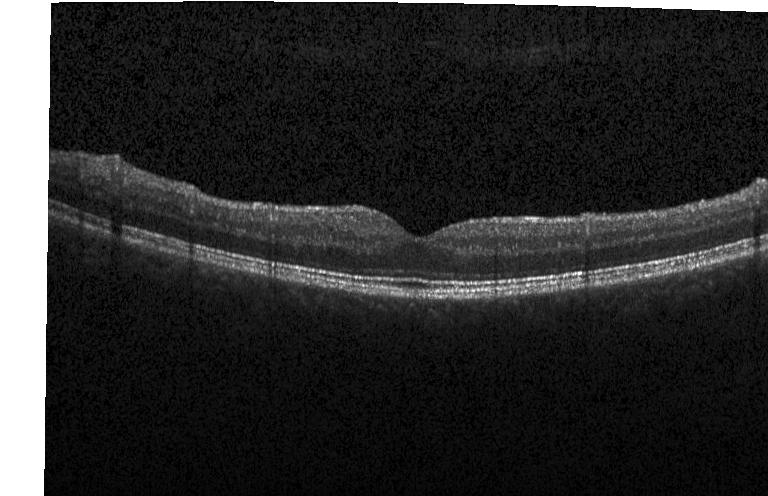
Impression: no choroidal neovascularization, diabetic macular edema, or drusen.